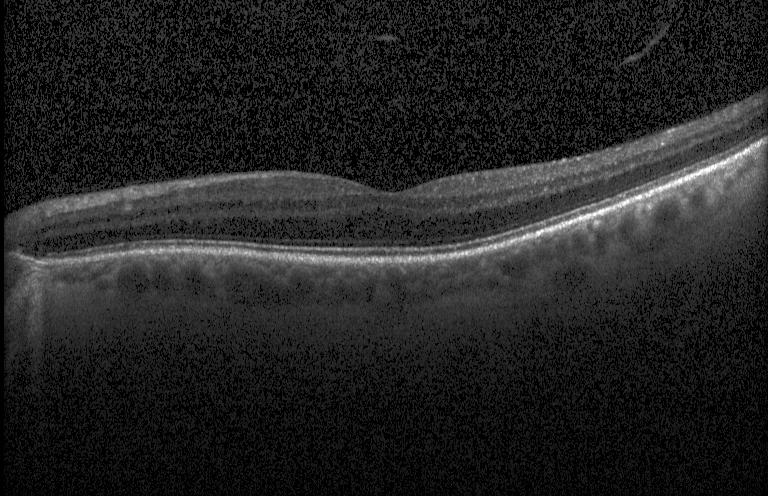
OCT B-scan.
This B-scan demonstrates neither choroidal neovascularization, diabetic macular edema, nor drusen.